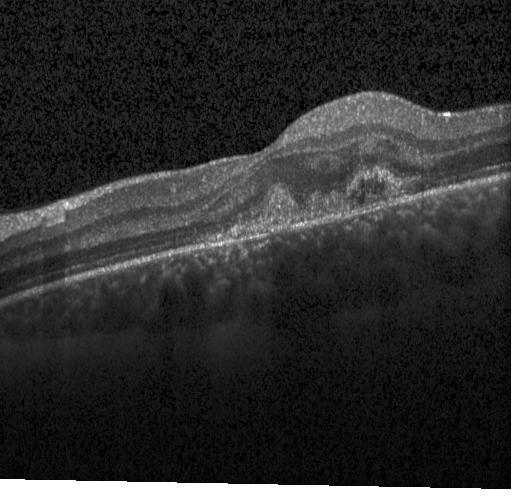

Horizontal scan through the fovea · OCT B-scan · spectral-domain optical coherence tomography.
OCT finding: choroidal neovascularization.